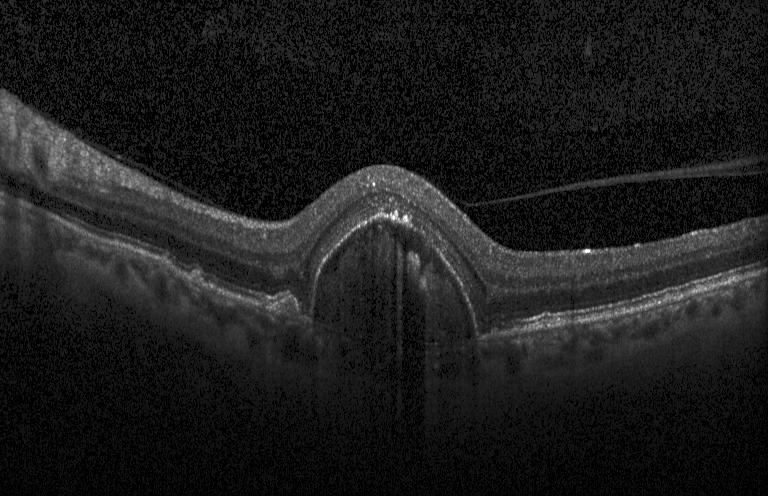 Fovea-centered · retinal OCT B-scan · Heidelberg Spectralis OCT system · spectral-domain OCT
This B-scan demonstrates CNV.